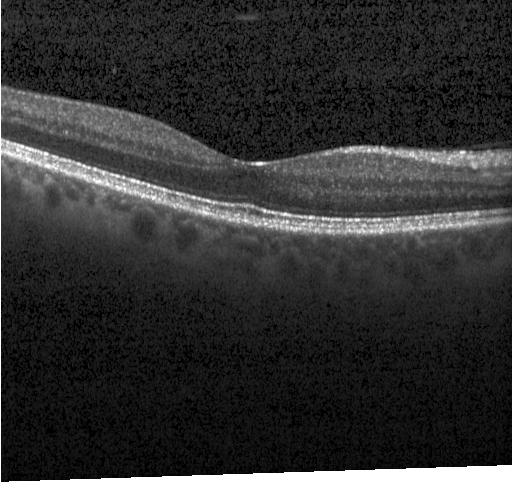

Impression: no choroidal neovascularization, diabetic macular edema, or drusen.